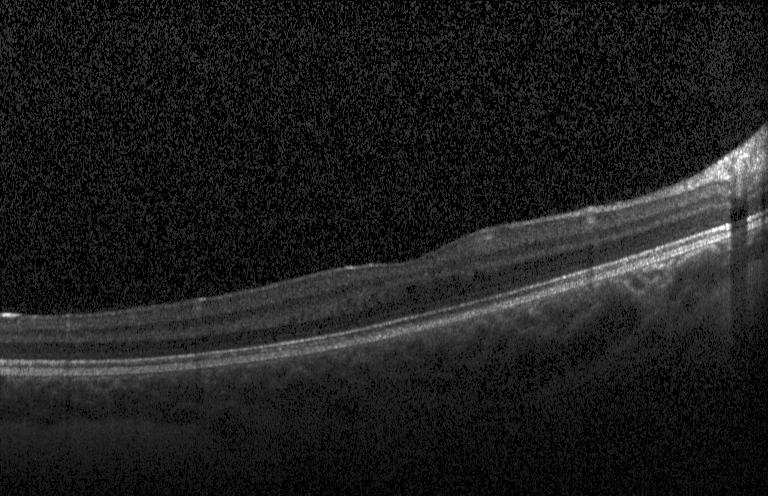

OCT line scan. Through the macula. Heidelberg Spectralis. SD-OCT — Diagnosis: no choroidal neovascularization, diabetic macular edema, or drusen.